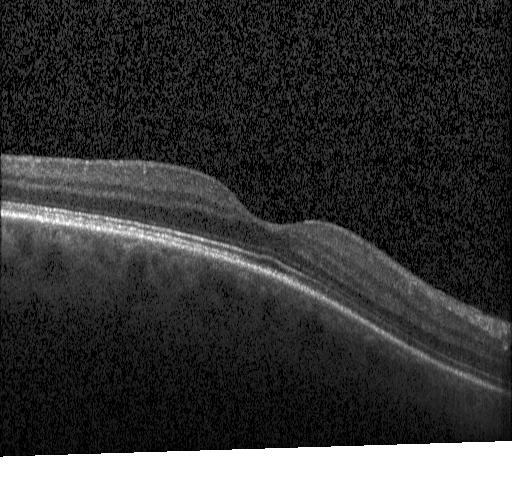
Acquired on a Heidelberg Spectralis. Centered on the fovea. Optical coherence tomography scan. Spectral-domain OCT.
Diagnosis: no CNV, DME, or drusen.